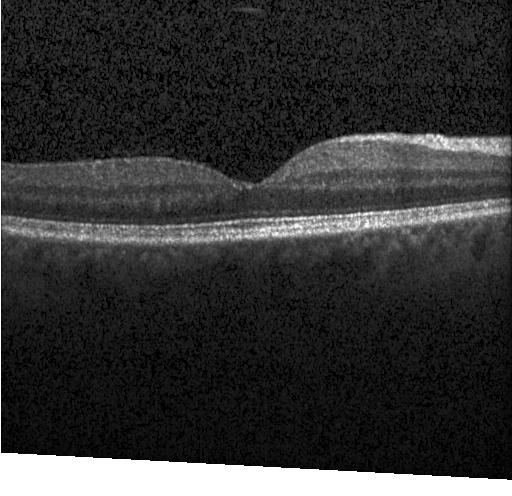

Retinal OCT B-scan. Finding: no evidence of choroidal neovascularization, diabetic macular edema, or drusen.